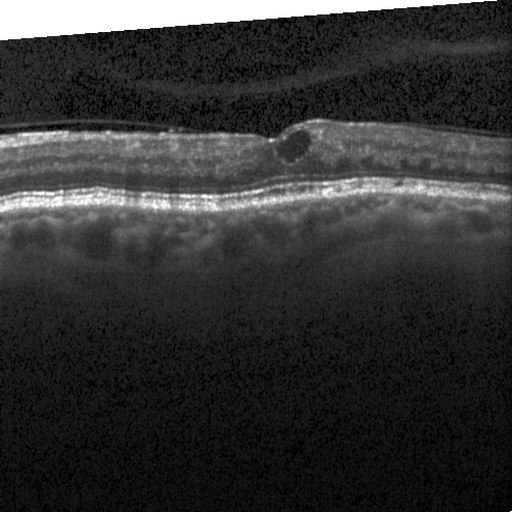 Heidelberg Spectralis; optical coherence tomography scan; SD-OCT
The scan shows diabetic macular edema.